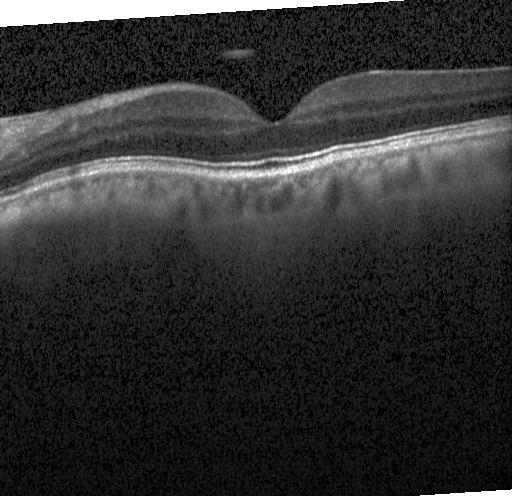 Optical coherence tomography B-scan; horizontal scan through the fovea.
Impression: no CNV, no DME, and no drusen.